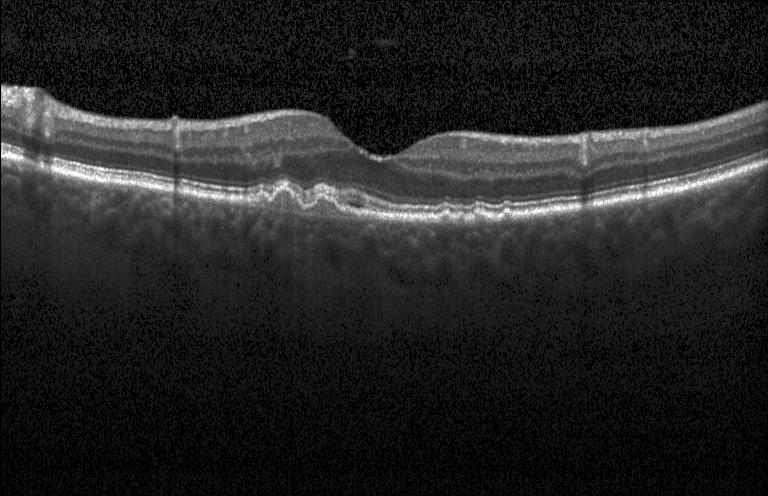

Optical coherence tomography B-scan.
Finding: a choroidal neovascular membrane.